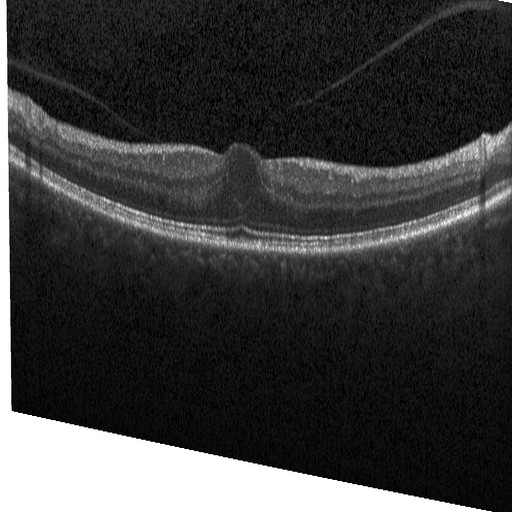 Through the macula; Heidelberg Spectralis OCT system; retinal OCT cross-section.
Dx: diabetic macular edema.